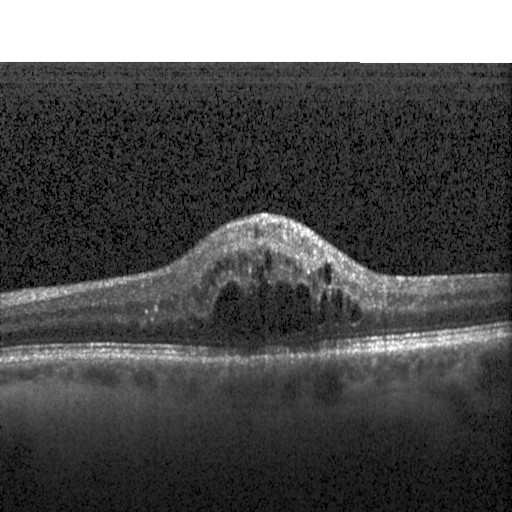 Optical coherence tomography scan. Acquired on a Heidelberg Spectralis. Fovea-centered. Spectral-domain OCT.
Impression: diabetic macular edema.